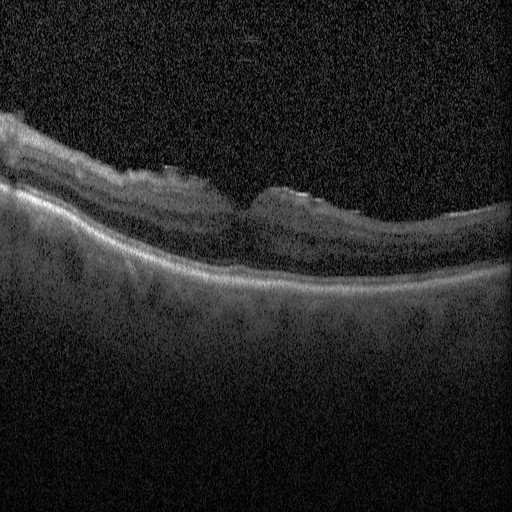 Dx: DME.